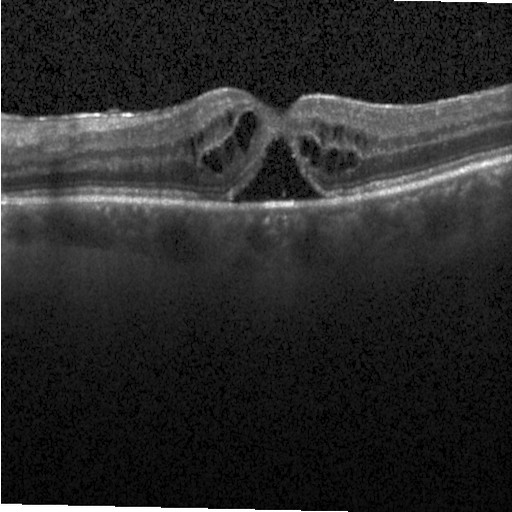
Optical coherence tomography scan. Spectral-domain OCT. OCT finding: DME.